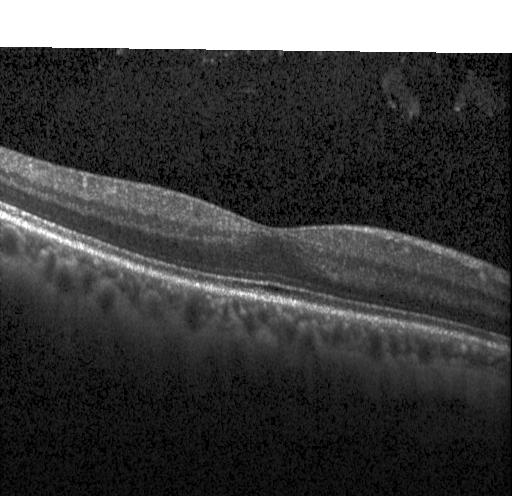
Finding: no CNV, DME, or drusen.